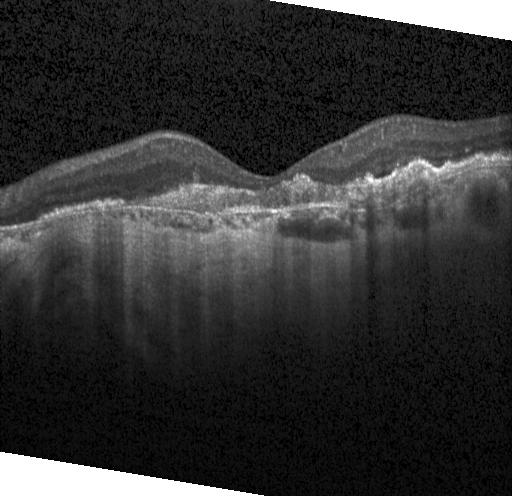
Impression: choroidal neovascularization (CNV).